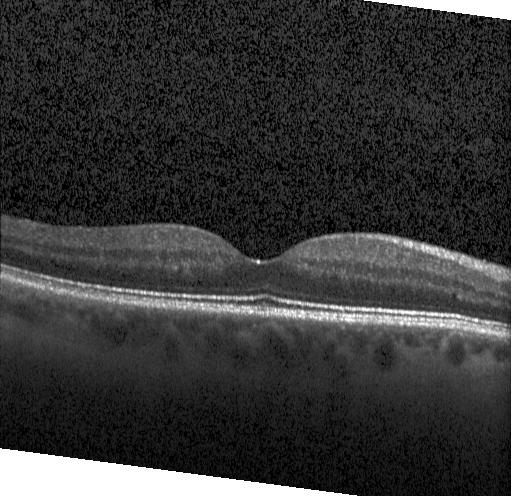
Optical coherence tomography B-scan.
Neither choroidal neovascularization, diabetic macular edema, nor drusen.